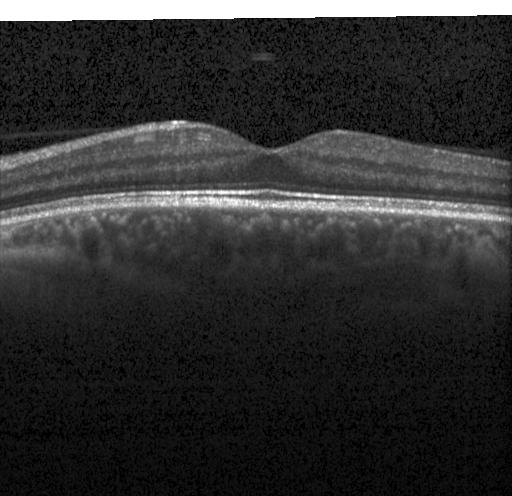

Retinal OCT cross-section · spectral-domain optical coherence tomography · horizontal scan through the fovea
This B-scan demonstrates no CNV, DME, or drusen.